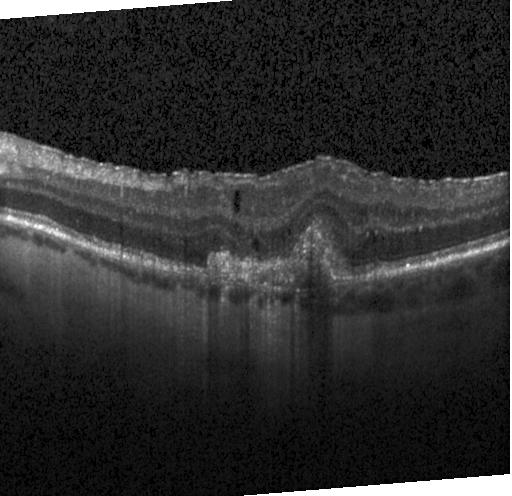
Optical coherence tomography B-scan
The scan shows a choroidal neovascular membrane.